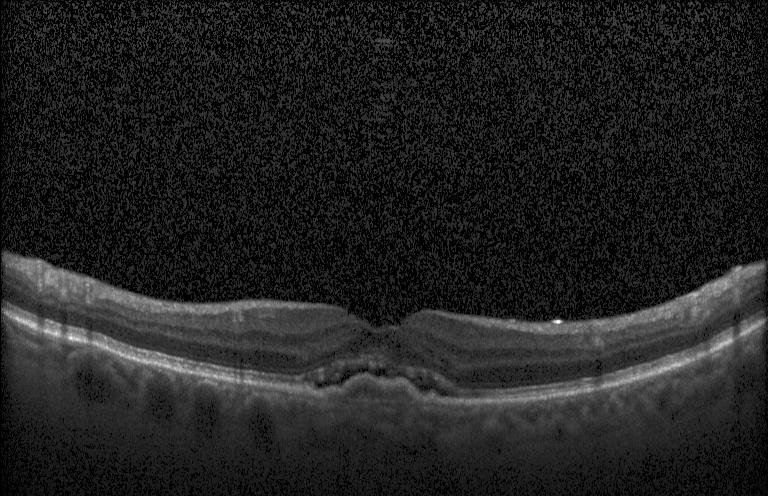
SD-OCT, instrument: Heidelberg Spectralis, retinal OCT B-scan, centered on the fovea. Impression: CNV.